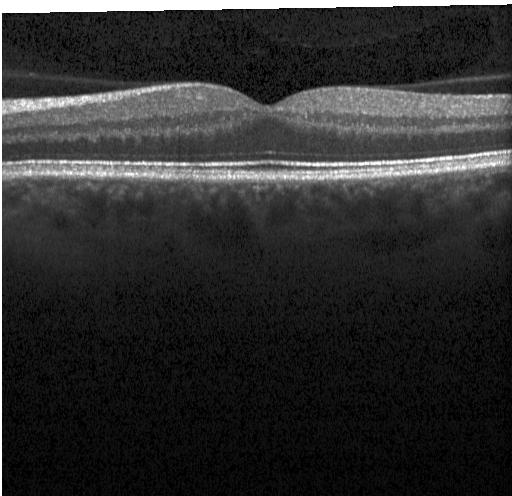
Centered on the fovea. SD-OCT. OCT B-scan — Diagnosis: no choroidal neovascularization, diabetic macular edema, or drusen.